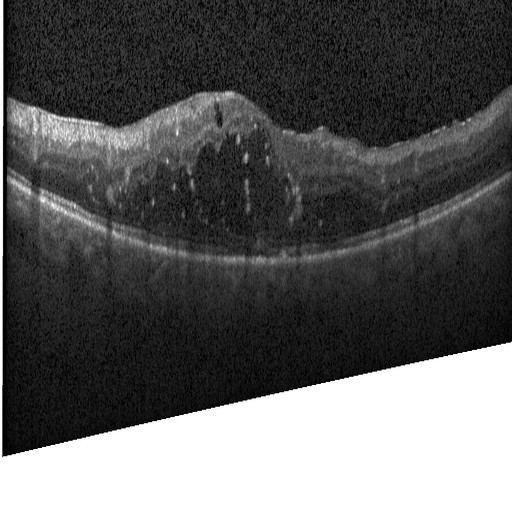

Finding: diabetic macular edema (DME).